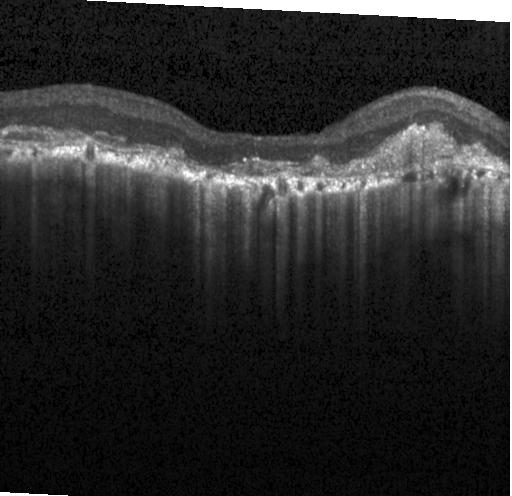 Retinal OCT cross-section. Finding: CNV.